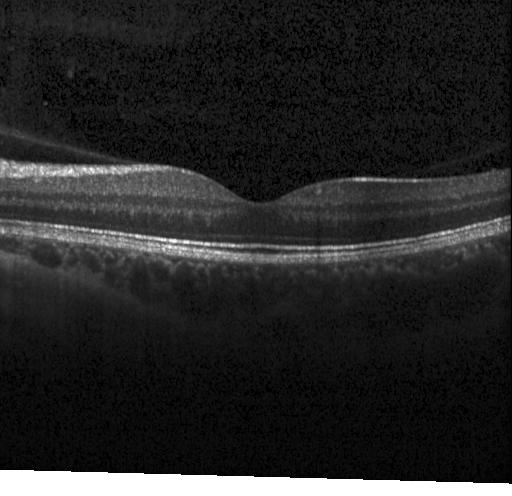 Instrument: Heidelberg Spectralis, spectral-domain OCT, OCT B-scan
Dx: neither CNV, DME, nor drusen.